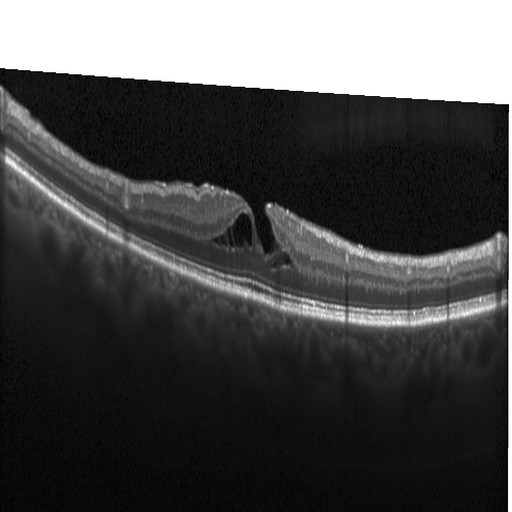
Through the macula; Heidelberg Spectralis; OCT line scan. Impression: DME.